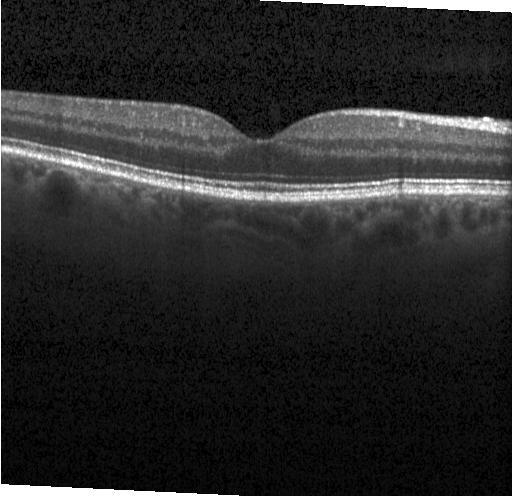

Macular scan, retinal OCT B-scan. The scan shows neither choroidal neovascularization, diabetic macular edema, nor drusen.